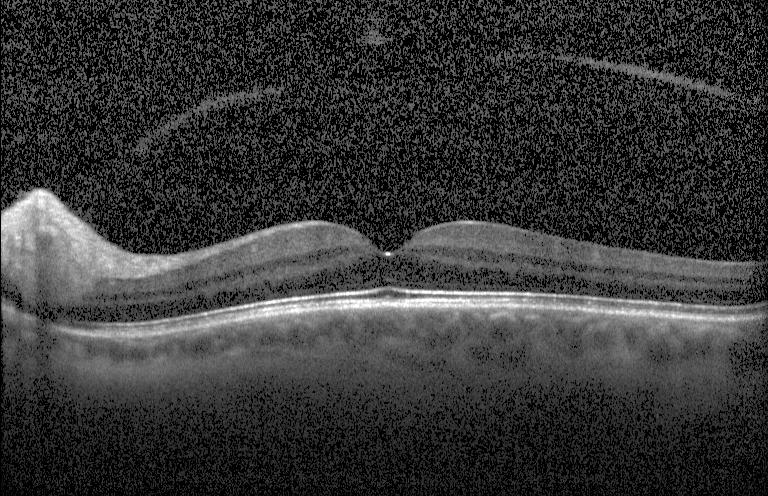 Fovea-centered. OCT line scan. OCT finding: no choroidal neovascularization, diabetic macular edema, or drusen.